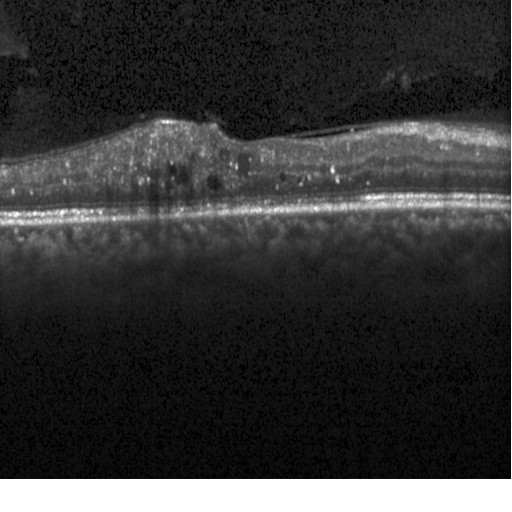

OCT scan showing DME.